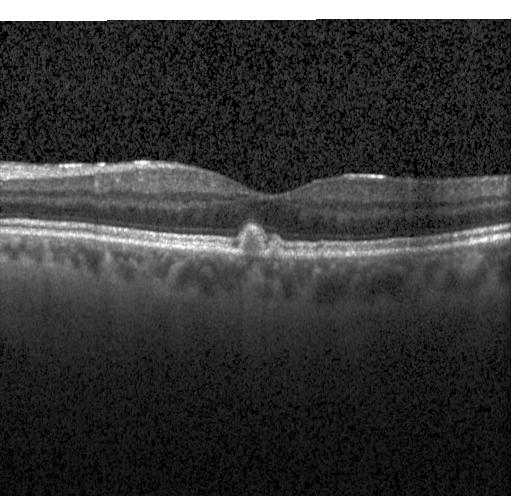

SD-OCT · OCT B-scan. Finding: drusen.